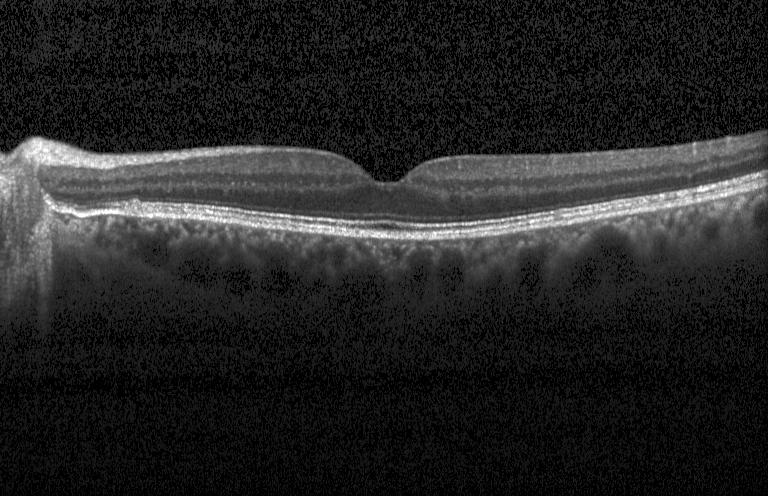 OCT finding: no choroidal neovascularization, no diabetic macular edema, and no drusen.